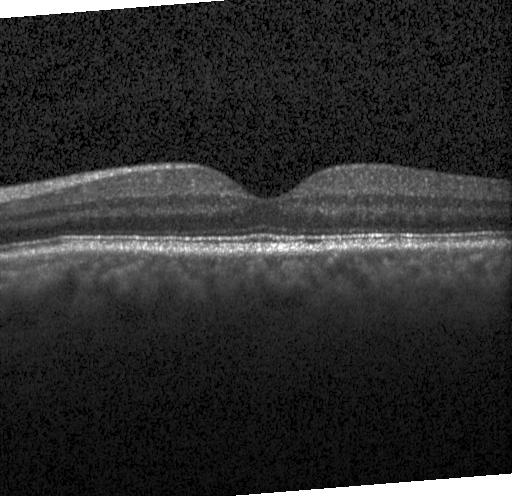
Spectral-domain OCT · OCT line scan · acquired on a Heidelberg Spectralis.
Dx: no evidence of choroidal neovascularization, diabetic macular edema, or drusen.